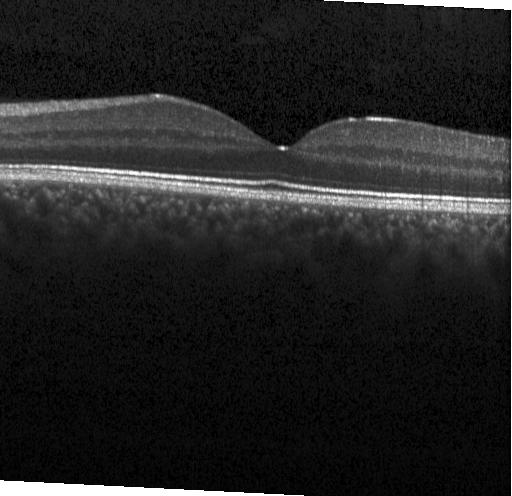

Diagnosis: no choroidal neovascularization, no diabetic macular edema, and no drusen.